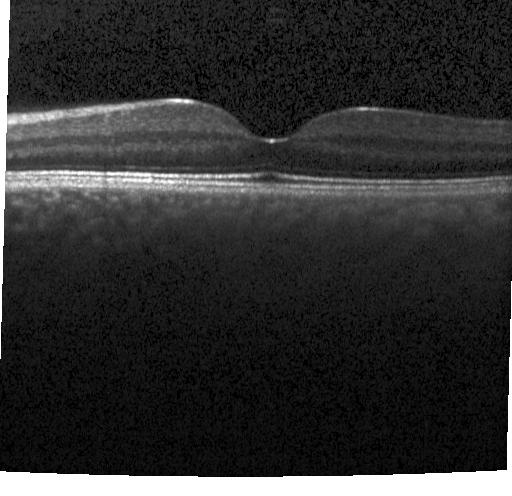

Heidelberg Spectralis. OCT B-scan
Impression: no choroidal neovascularization, no diabetic macular edema, and no drusen.